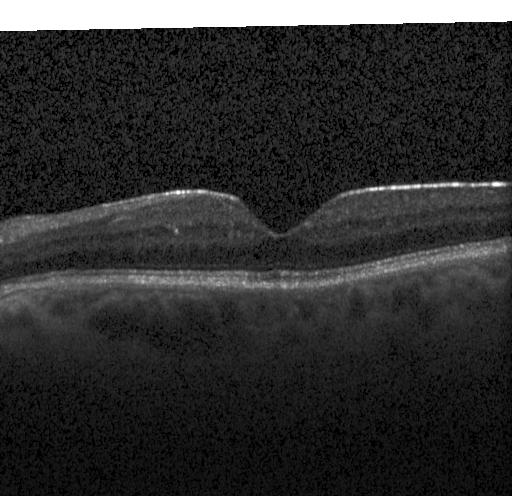
Impression: no CNV, DME, or drusen.